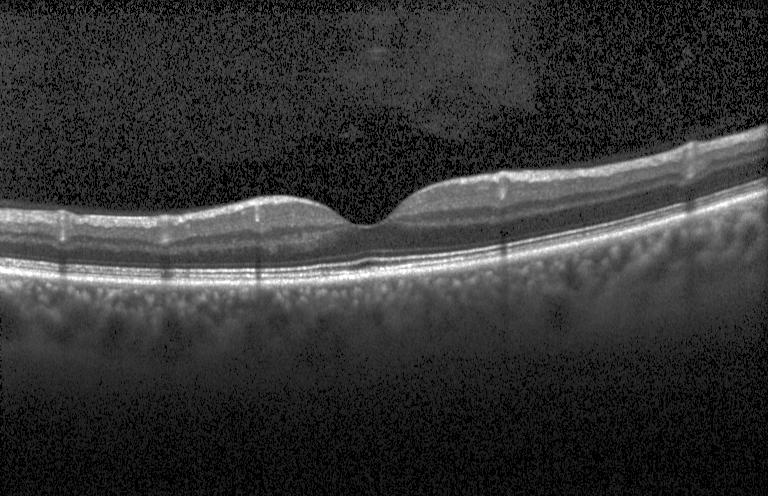

Spectral-domain OCT; OCT line scan; Heidelberg Spectralis
Impression: no evidence of choroidal neovascularization, diabetic macular edema, or drusen.